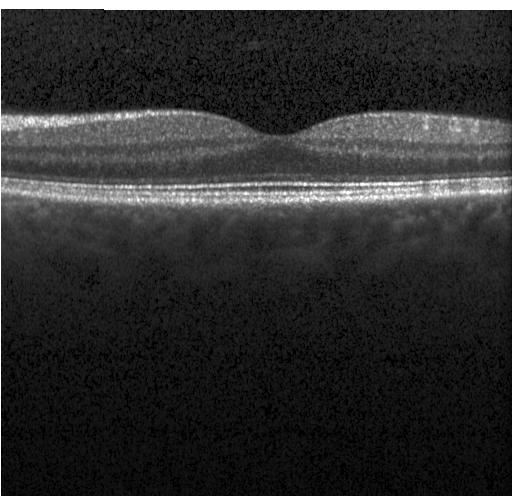
Retinal OCT B-scan.
Impression: no choroidal neovascularization, no diabetic macular edema, and no drusen.